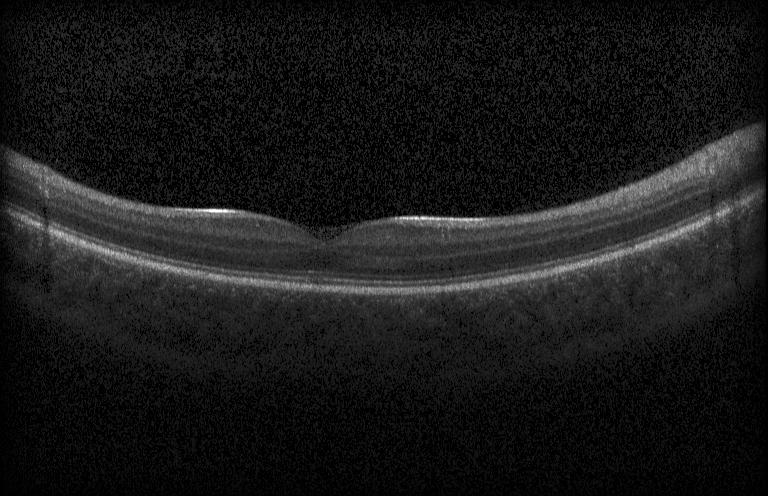 Diagnosis: neither choroidal neovascularization, diabetic macular edema, nor drusen.